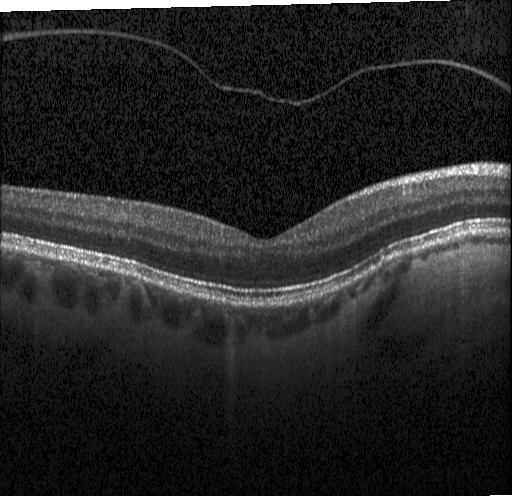

OCT line scan — The scan shows no choroidal neovascularization, diabetic macular edema, or drusen.